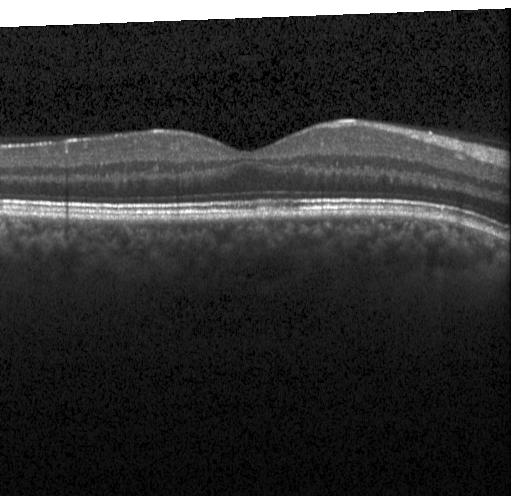

OCT B-scan, acquired on a Heidelberg Spectralis, macular scan, spectral-domain OCT. Diagnosis: no CNV, no DME, and no drusen.